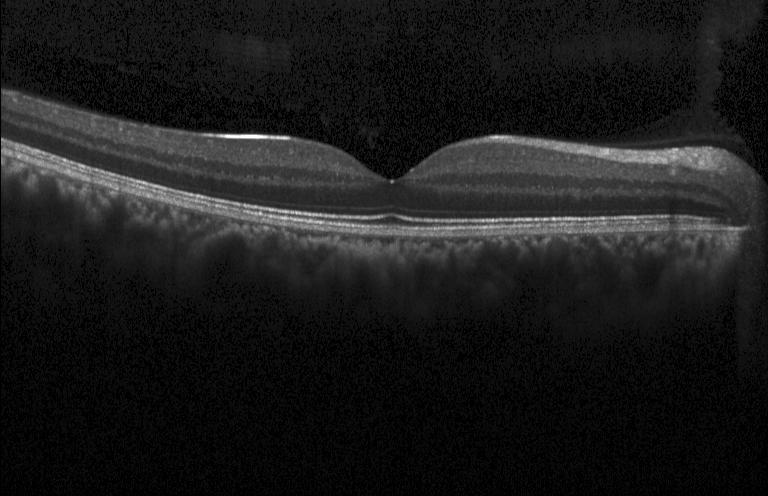 SD-OCT; retinal OCT cross-section. Assessment: no choroidal neovascularization, diabetic macular edema, or drusen.